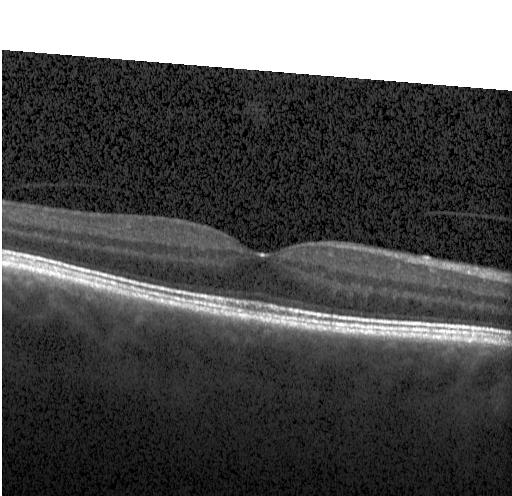 Diagnosis: neither CNV, DME, nor drusen.